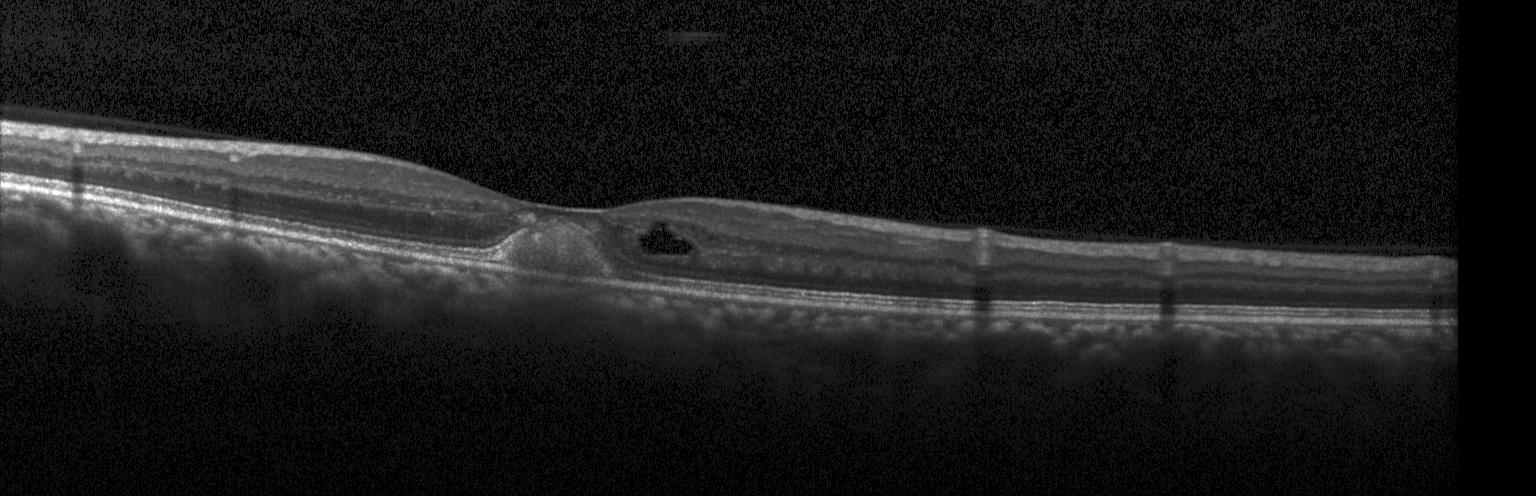
Optical coherence tomography scan — OCT finding: a choroidal neovascular membrane.